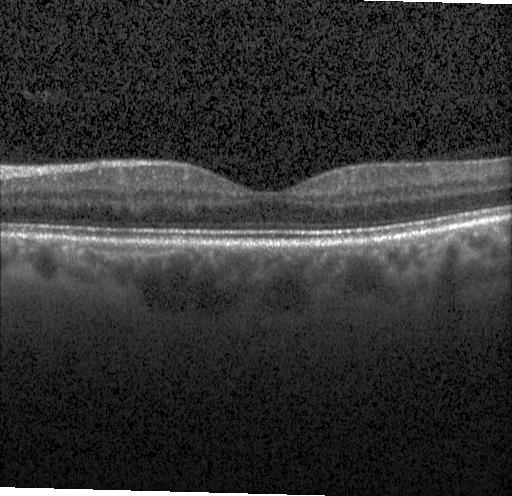
Instrument: Heidelberg Spectralis, retinal OCT B-scan. No CNV, DME, or drusen.